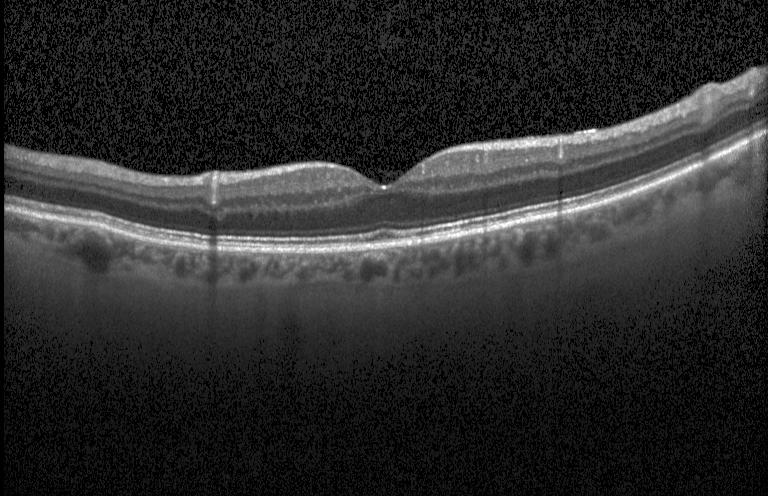

Retinal OCT B-scan. Fovea-centered. Acquired on a Heidelberg Spectralis. Spectral-domain OCT. This B-scan demonstrates no choroidal neovascularization, diabetic macular edema, or drusen.